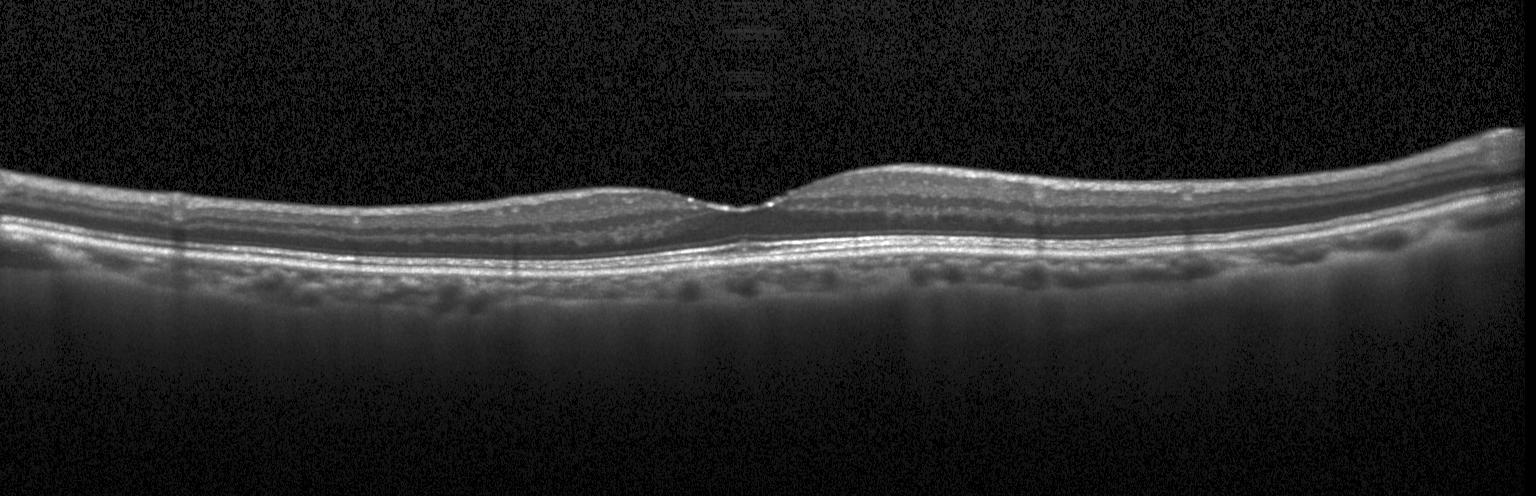 Spectral-domain OCT. OCT B-scan
Dx: no CNV, DME, or drusen.